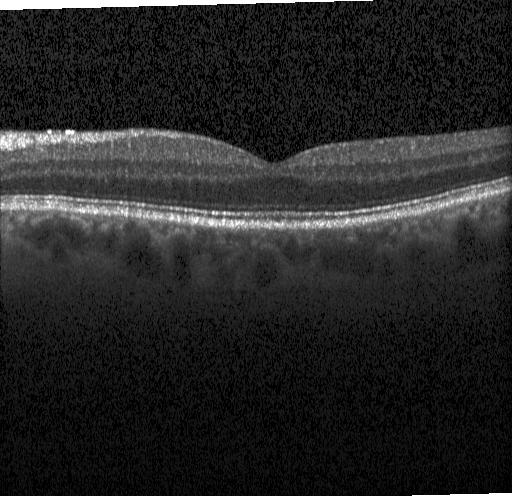 Macular OCT: no CNV, DME, or drusen.